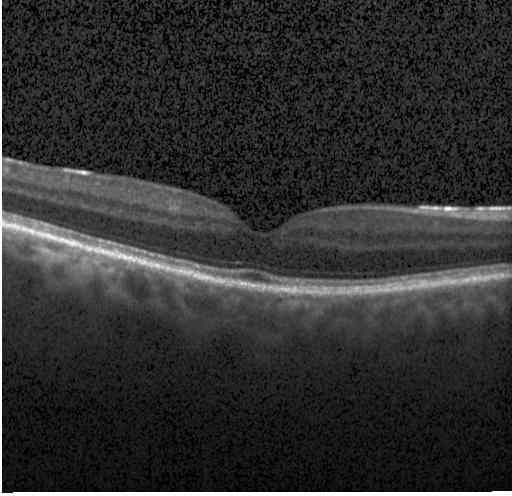 Retinal OCT cross-section showing no CNV, no DME, and no drusen.